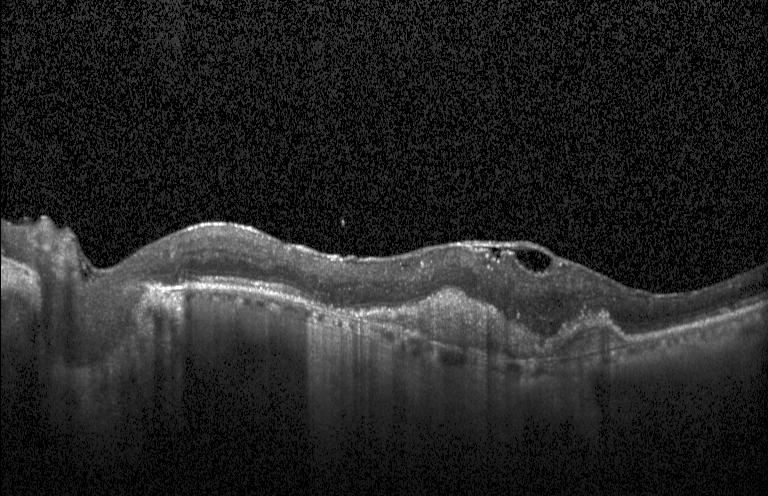
Finding: a choroidal neovascular membrane.